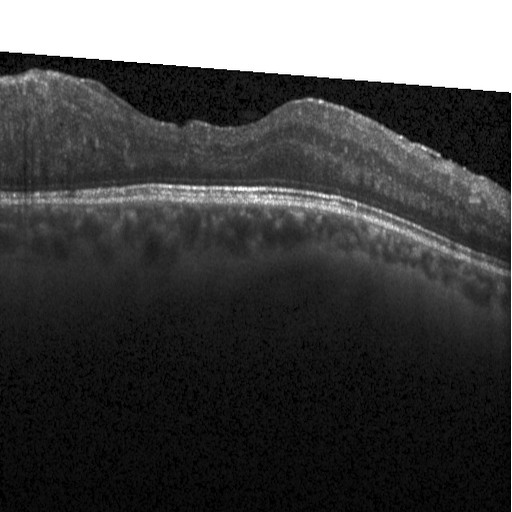 Finding: diabetic macular edema.